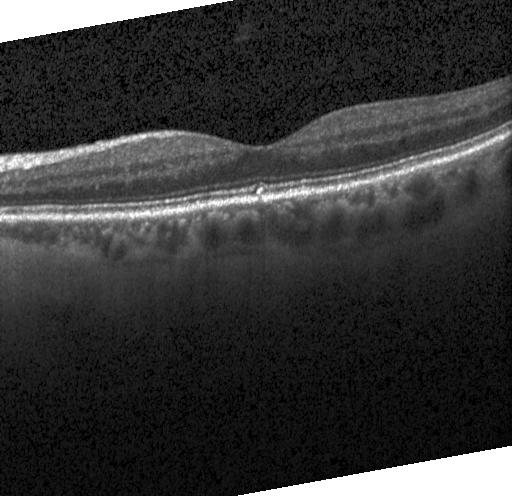

OCT B-scan showing no evidence of CNV, DME, or drusen.